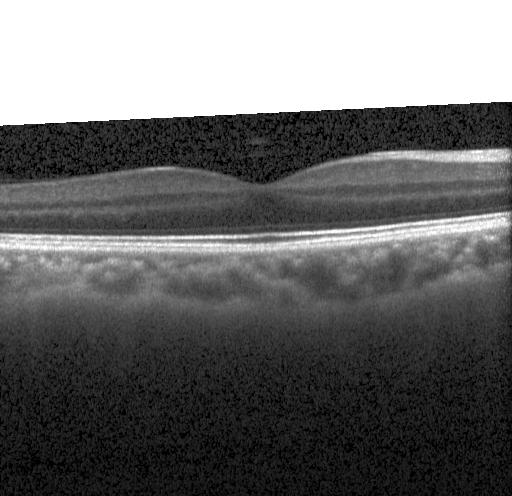 Assessment: no evidence of choroidal neovascularization, diabetic macular edema, or drusen.